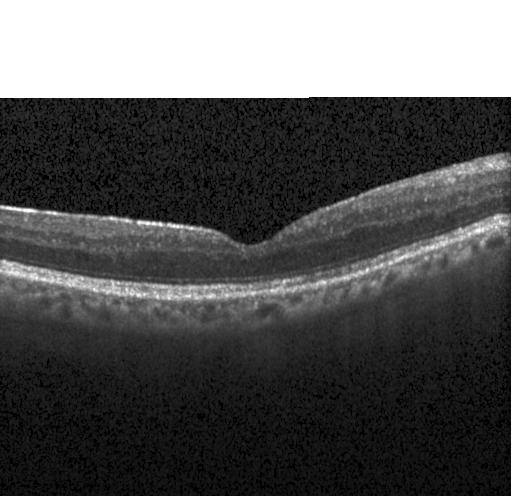 OCT finding: no CNV, no DME, and no drusen.